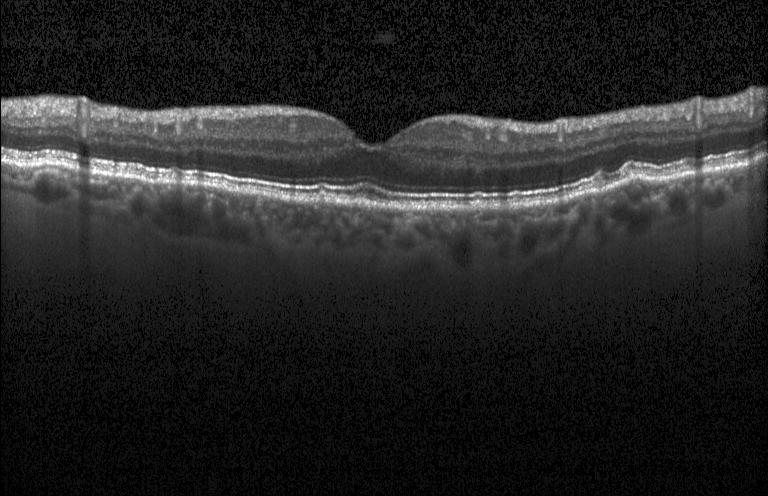

Retinal OCT cross-section. Diagnosis: sub-RPE drusenoid deposits.